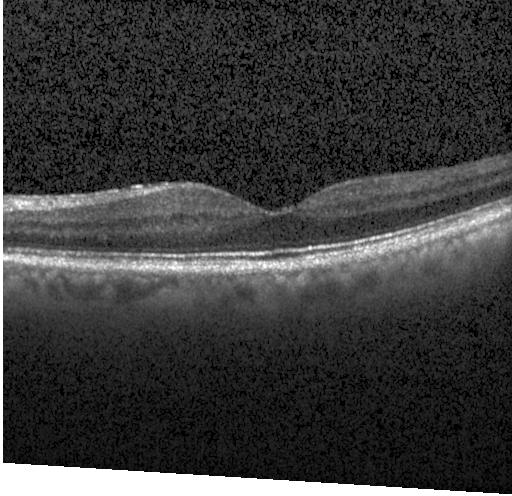
Macular scan, instrument: Heidelberg Spectralis, optical coherence tomography scan — Macular OCT: neither CNV, DME, nor drusen.